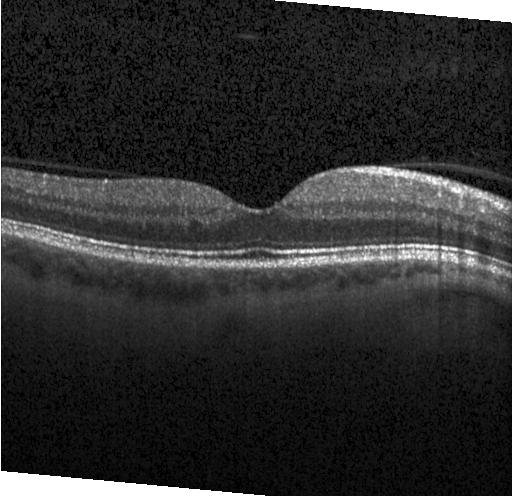 Optical coherence tomography B-scan
Assessment: no choroidal neovascularization, diabetic macular edema, or drusen.